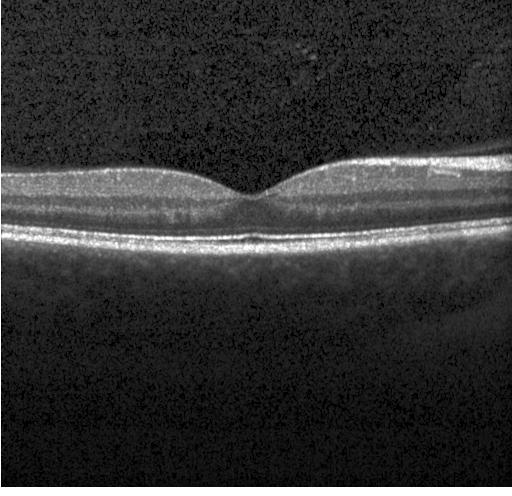

Macular scan. OCT line scan. Spectral-domain optical coherence tomography. Dx: neither choroidal neovascularization, diabetic macular edema, nor drusen.